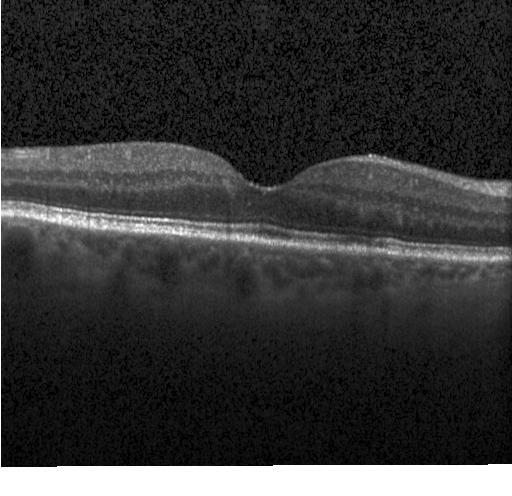 Finding: no choroidal neovascularization, diabetic macular edema, or drusen.